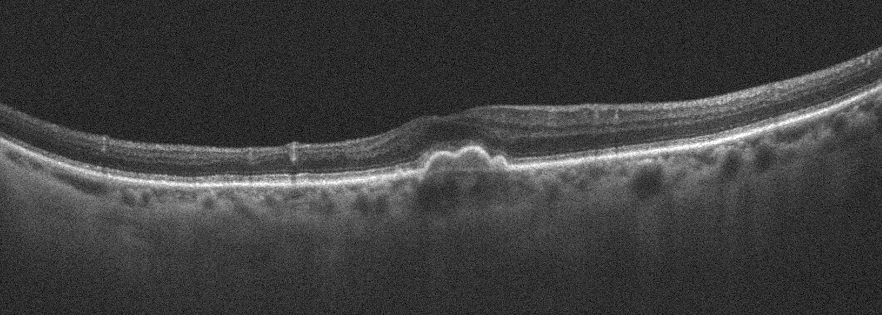

OCT B-scan · OD.
Impression: age-related macular degeneration (AMD).